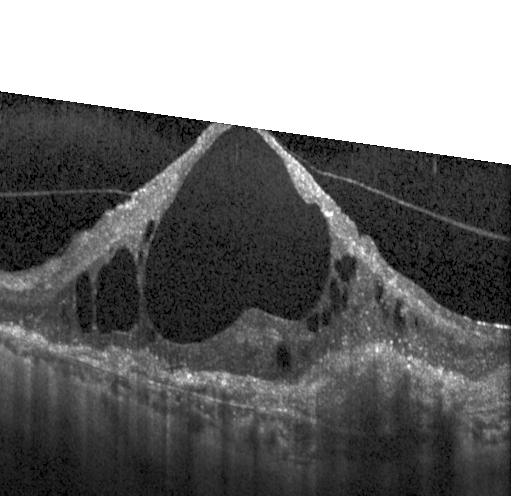

Spectral-domain optical coherence tomography · instrument: Heidelberg Spectralis · through the macula · OCT line scan.
Finding: CNV.